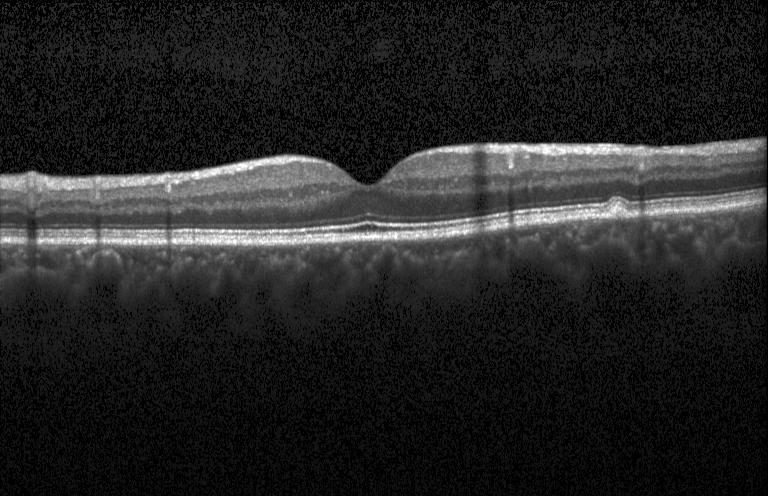
Optical coherence tomography scan, fovea-centered, Heidelberg Spectralis OCT system
Assessment: sub-RPE drusenoid deposits.